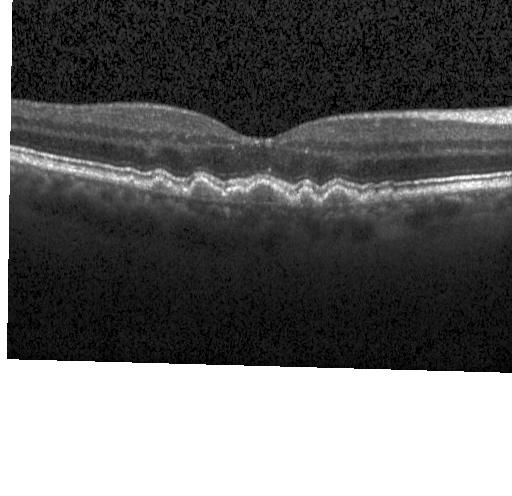

OCT line scan. This B-scan demonstrates drusen.